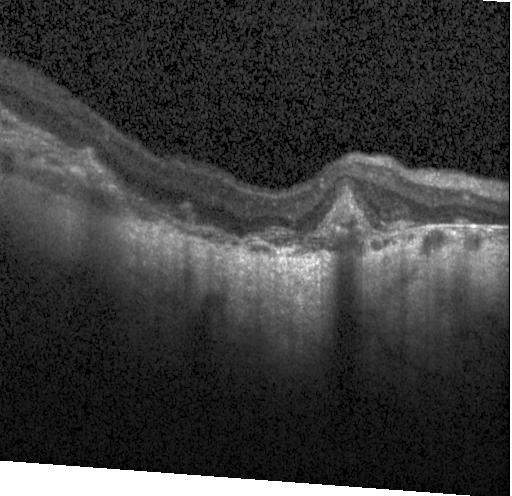 Macular OCT: choroidal neovascularization (CNV).